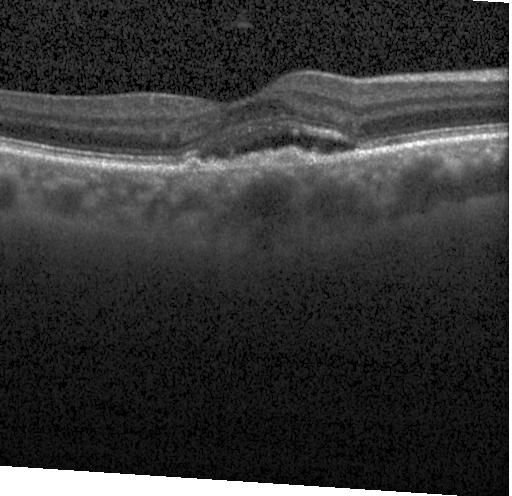 Retinal OCT B-scan, macular scan, Heidelberg Spectralis OCT system.
This B-scan demonstrates CNV.